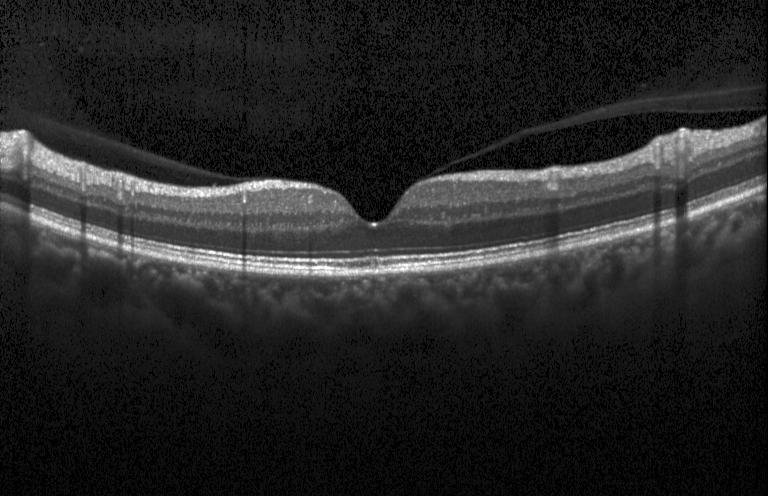 Finding: neither choroidal neovascularization, diabetic macular edema, nor drusen.